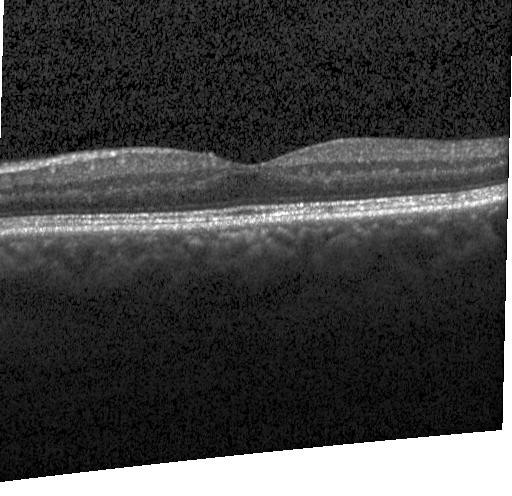 Dx: no evidence of choroidal neovascularization, diabetic macular edema, or drusen.